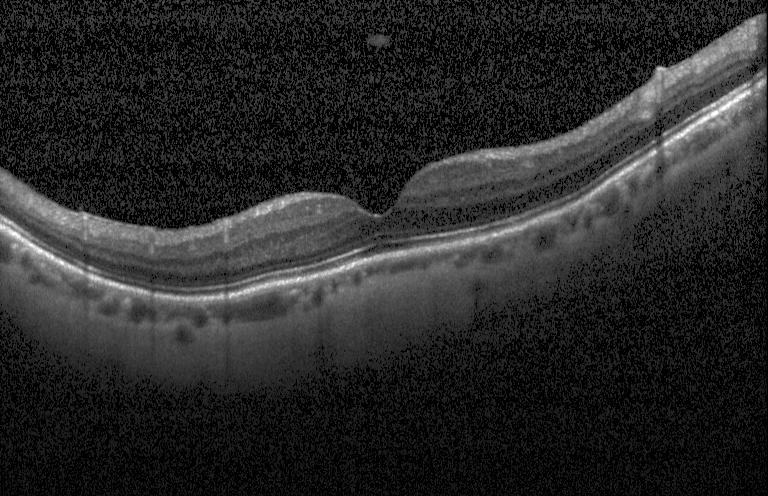

Acquired on a Heidelberg Spectralis; optical coherence tomography B-scan.
Finding: no evidence of choroidal neovascularization, diabetic macular edema, or drusen.